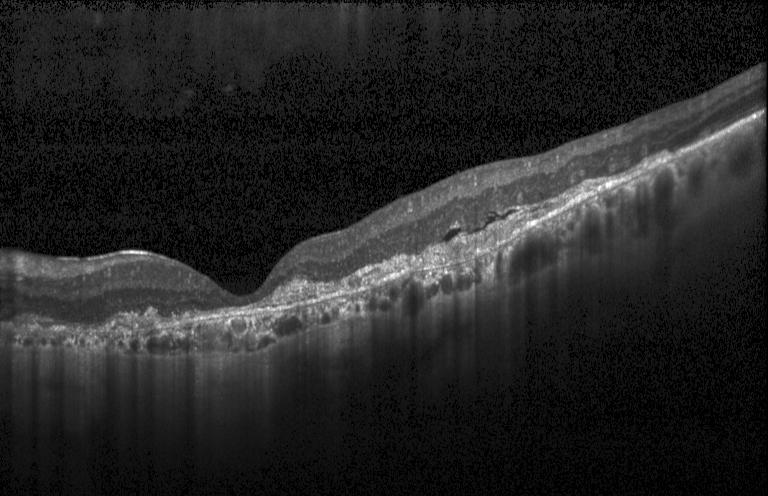 Macular OCT demonstrating a choroidal neovascular membrane.